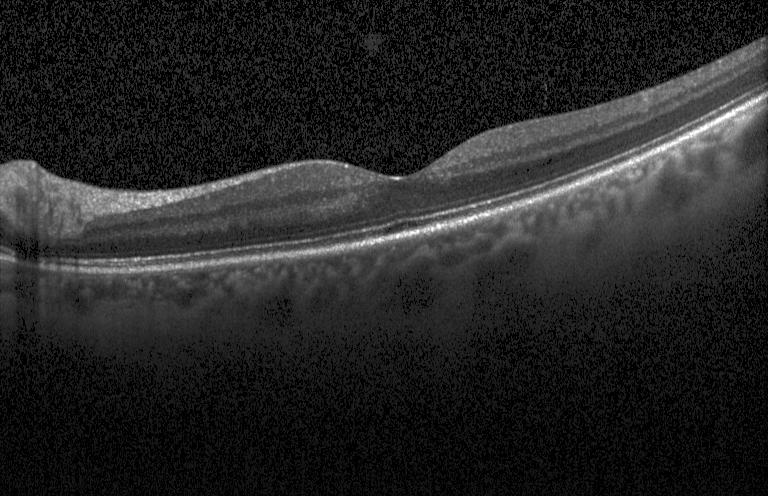 Impression: no CNV, DME, or drusen.